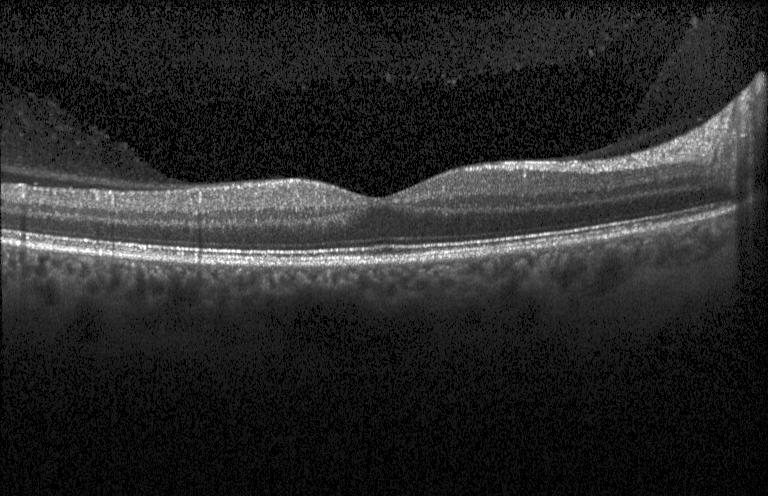 Heidelberg Spectralis · retinal OCT cross-section · spectral-domain OCT — This B-scan demonstrates no choroidal neovascularization, no diabetic macular edema, and no drusen.